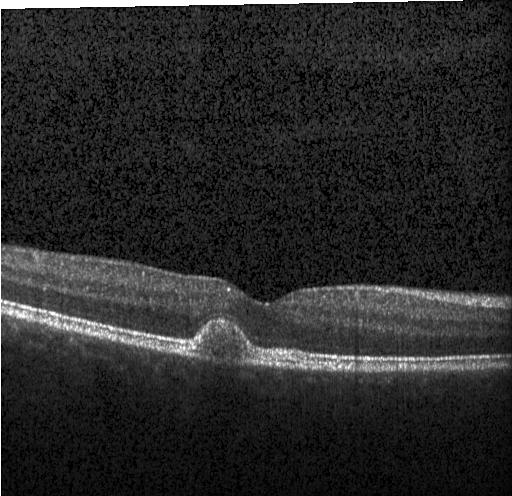 Heidelberg Spectralis OCT system; optical coherence tomography scan; through the macula; SD-OCT — OCT finding: sub-RPE drusenoid deposits.